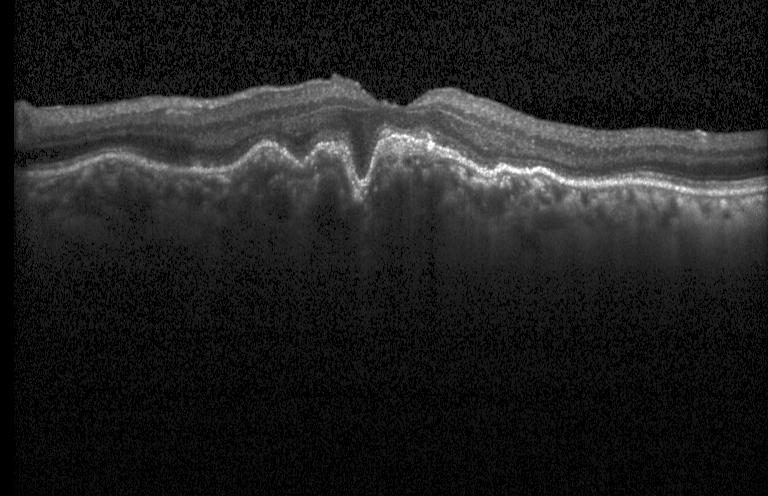
Assessment: a choroidal neovascular membrane.